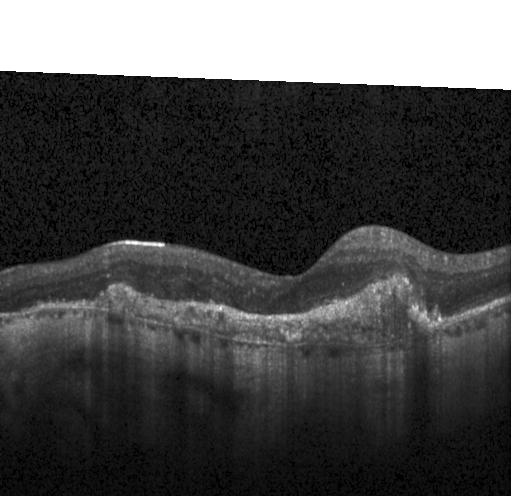 Heidelberg Spectralis OCT system · spectral-domain OCT · fovea-centered · OCT B-scan. OCT finding: a choroidal neovascular membrane.